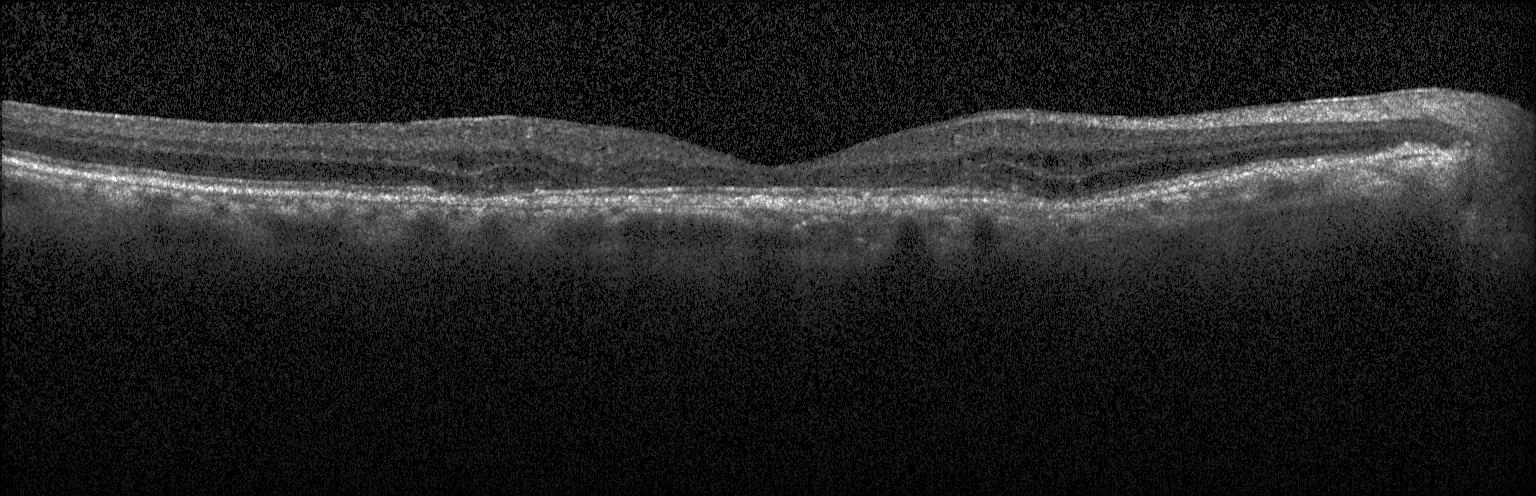

Acquired on a Heidelberg Spectralis · retinal OCT B-scan · centered on the fovea · spectral-domain optical coherence tomography. Finding: a choroidal neovascular membrane.